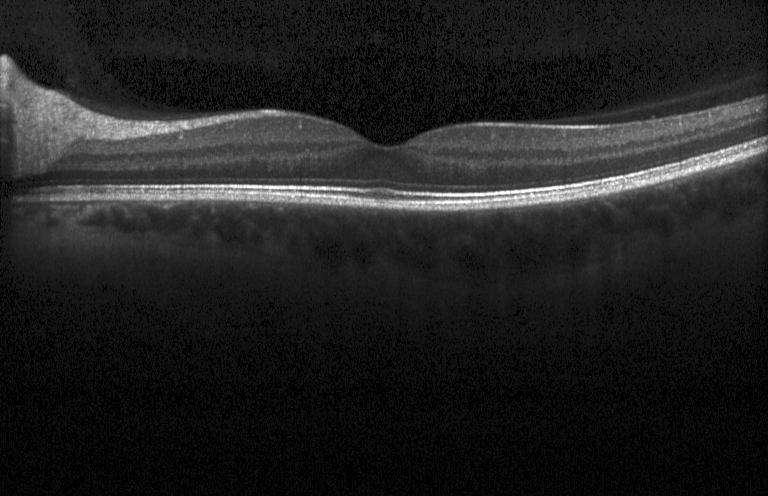

Spectral-domain OCT B-scan: no choroidal neovascularization, no diabetic macular edema, and no drusen.